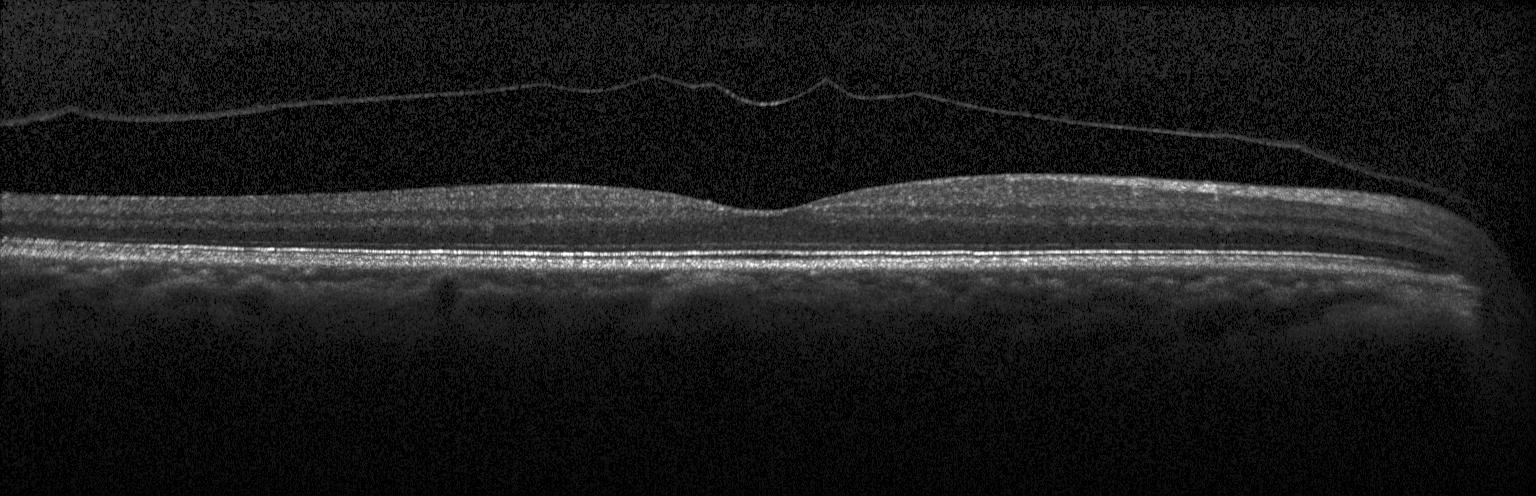
Finding: no CNV, no DME, and no drusen.